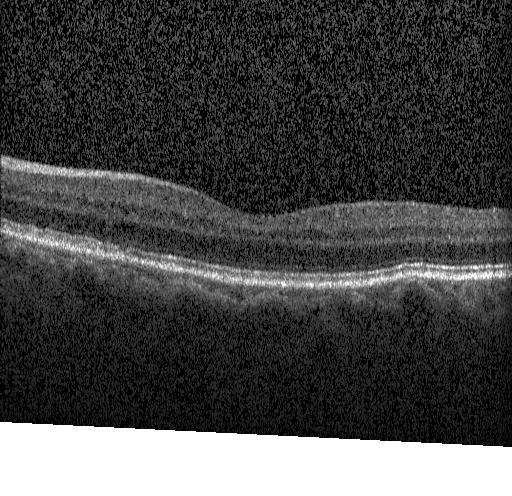
Retinal OCT cross-section — Diagnosis: multiple drusen.